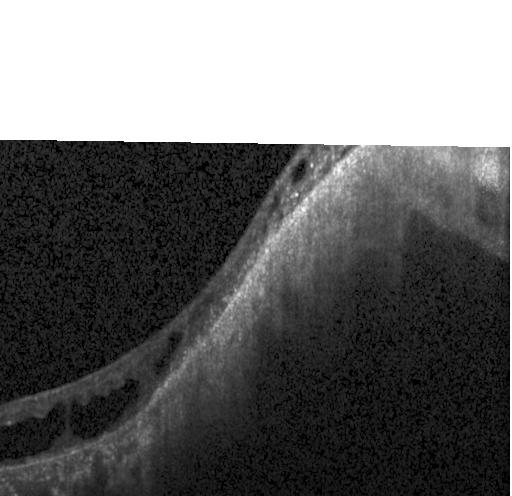
Retinal OCT B-scan — Diagnosis: diabetic macular edema.